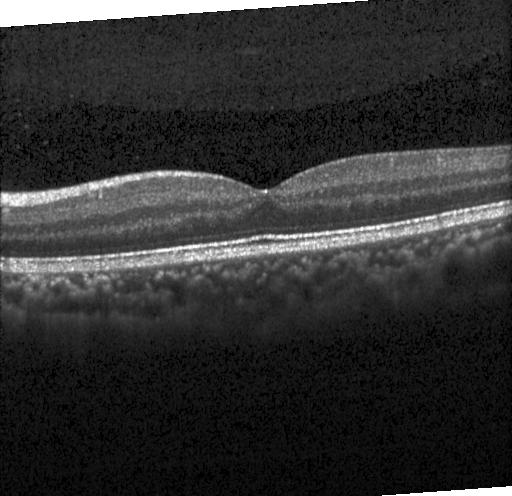

Fovea-centered. Spectral-domain optical coherence tomography. Heidelberg Spectralis OCT system. OCT B-scan. Macular OCT: no CNV, DME, or drusen.